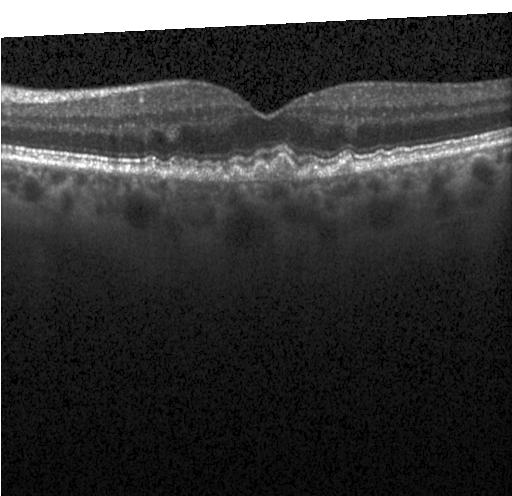 Multiple drusen.